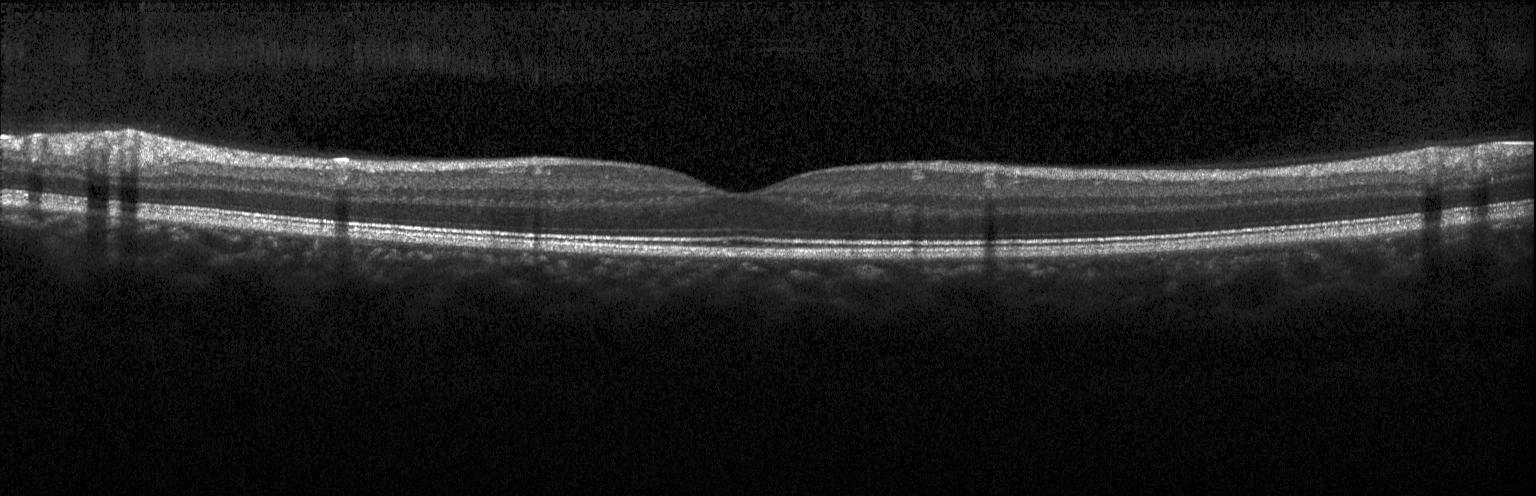

Macular scan; OCT line scan; Heidelberg Spectralis; spectral-domain optical coherence tomography. Macular OCT: no evidence of CNV, DME, or drusen.